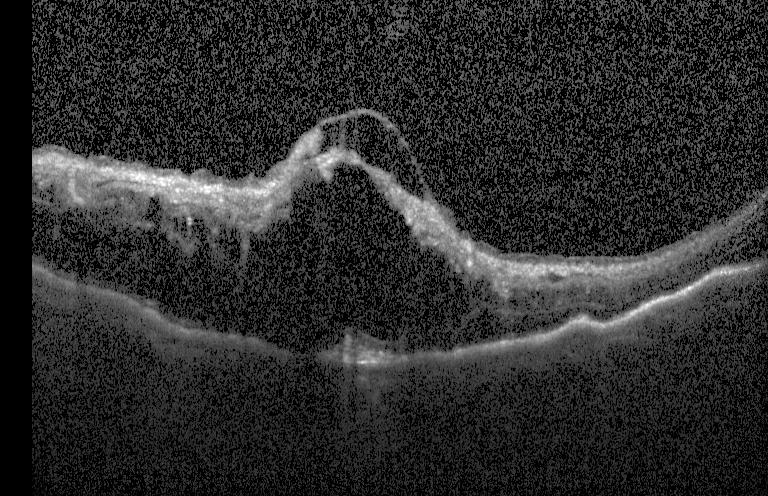
Retinal OCT cross-section. OCT finding: diabetic macular edema (DME).